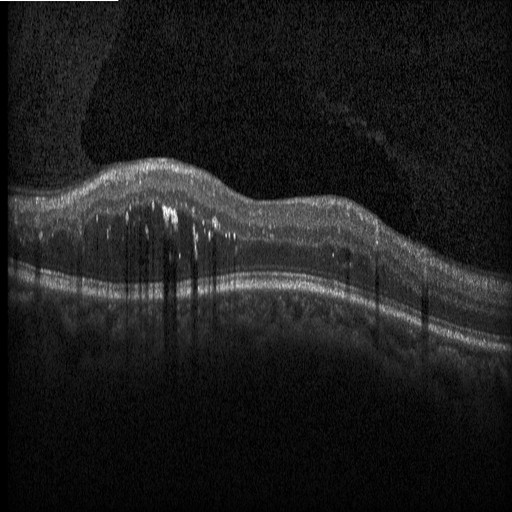

Impression: diabetic macular edema (DME).